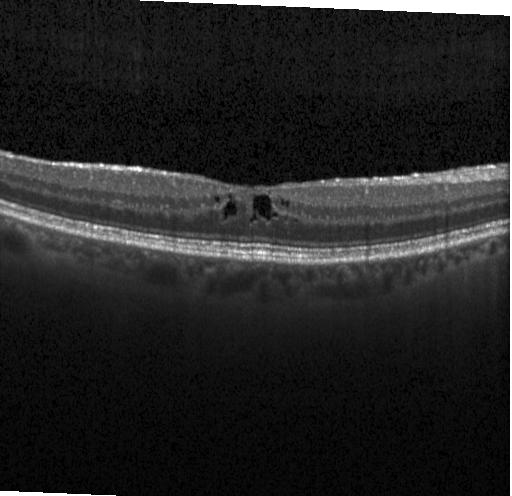

OCT B-scan · macular scan · SD-OCT · instrument: Heidelberg Spectralis — Diagnosis: diabetic macular edema.